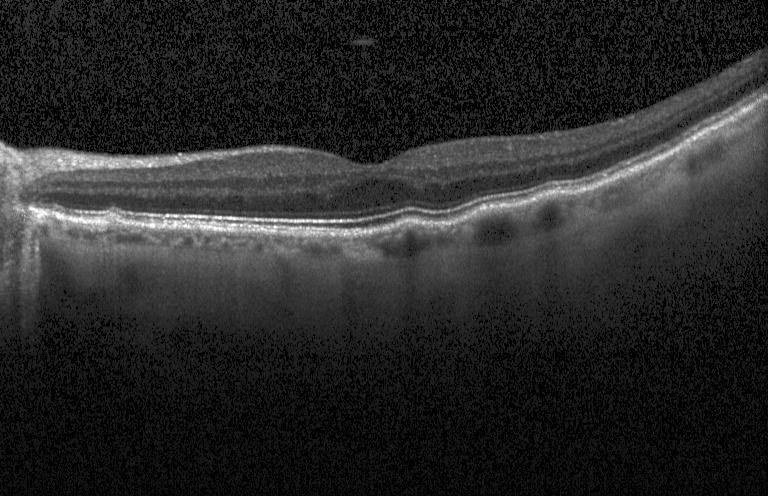 Retinal OCT cross-section showing no evidence of choroidal neovascularization, diabetic macular edema, or drusen.